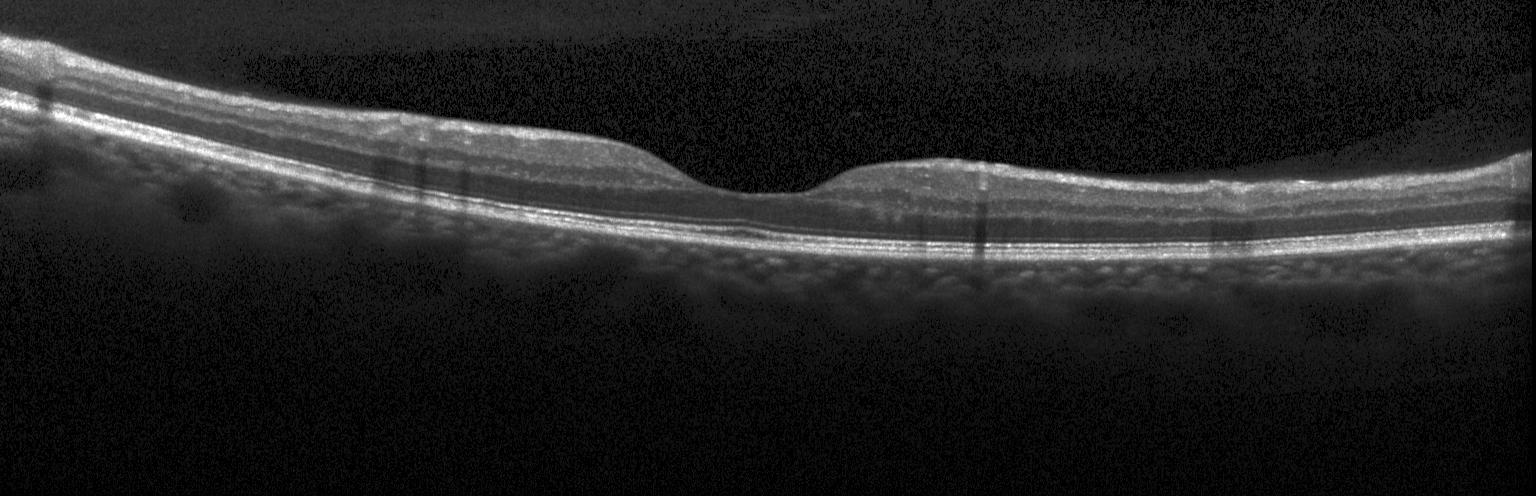 Acquired on a Heidelberg Spectralis, SD-OCT, macular scan, retinal OCT cross-section — Diagnosis: no choroidal neovascularization, diabetic macular edema, or drusen.